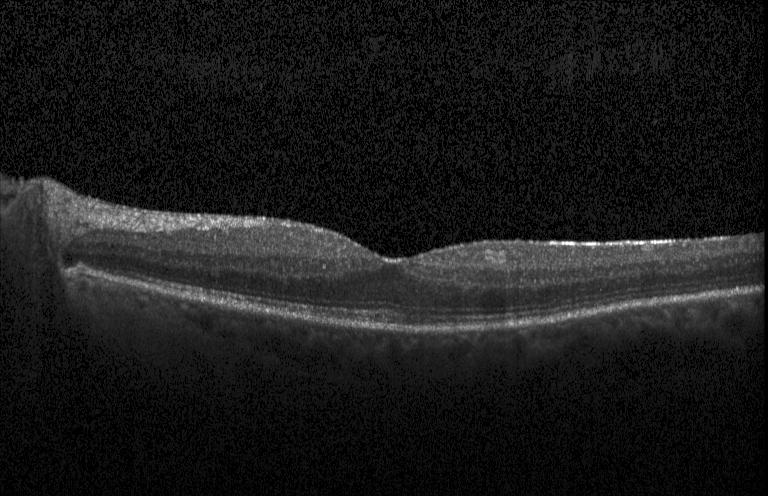

Macular OCT: neither choroidal neovascularization, diabetic macular edema, nor drusen.